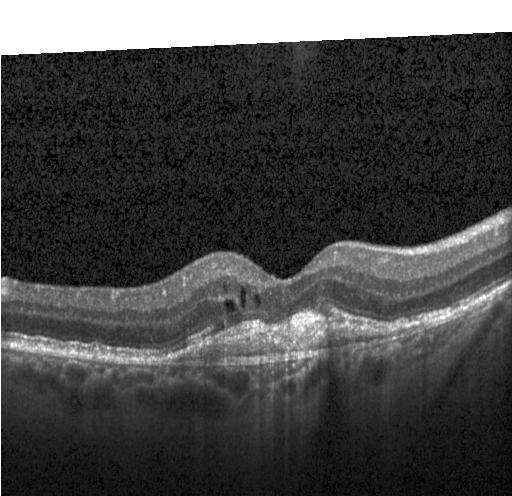 Dx: a choroidal neovascular membrane.